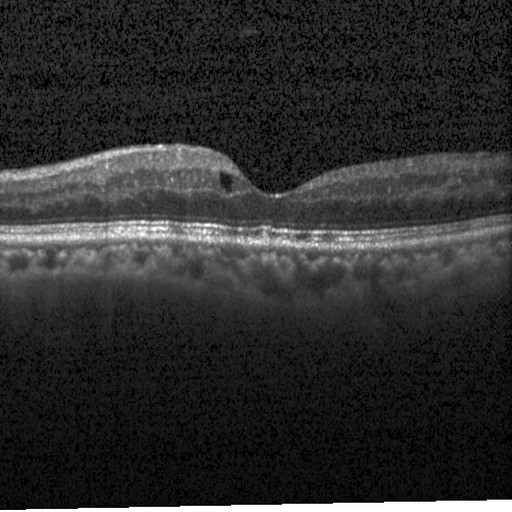

Macular scan; Heidelberg Spectralis; retinal OCT cross-section; spectral-domain optical coherence tomography
Impression: diabetic macular edema.